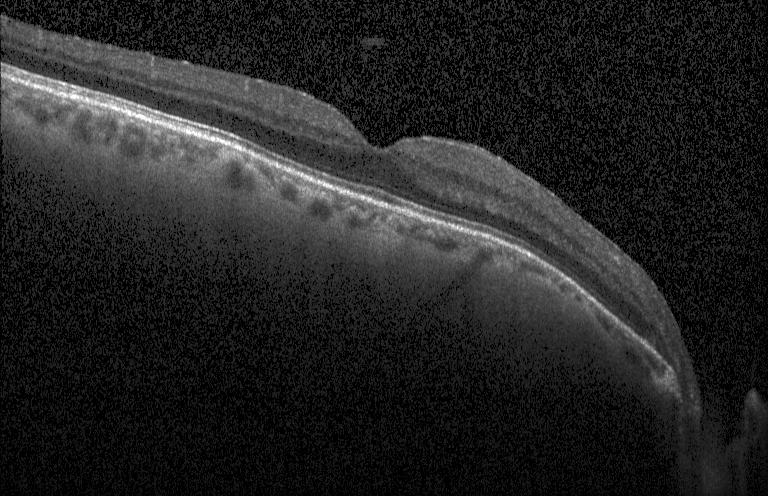

Acquired on a Heidelberg Spectralis. OCT B-scan. Fovea-centered. This B-scan demonstrates no choroidal neovascularization, no diabetic macular edema, and no drusen.